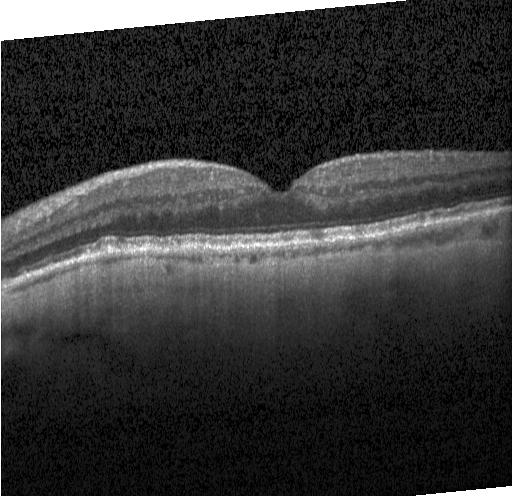

OCT B-scan.
Diagnosis: drusen.